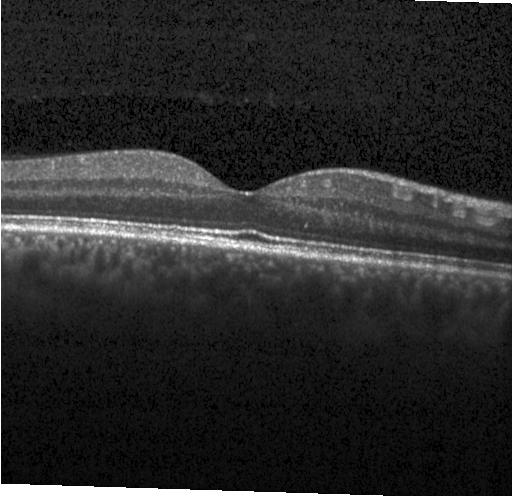
SD-OCT; OCT B-scan
This B-scan demonstrates no CNV, no DME, and no drusen.